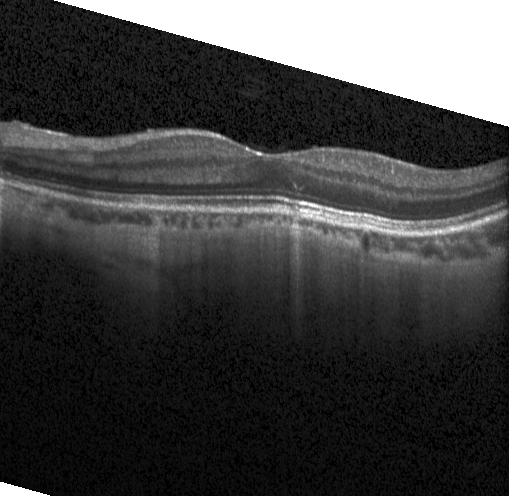

OCT B-scan — This B-scan demonstrates neither CNV, DME, nor drusen.